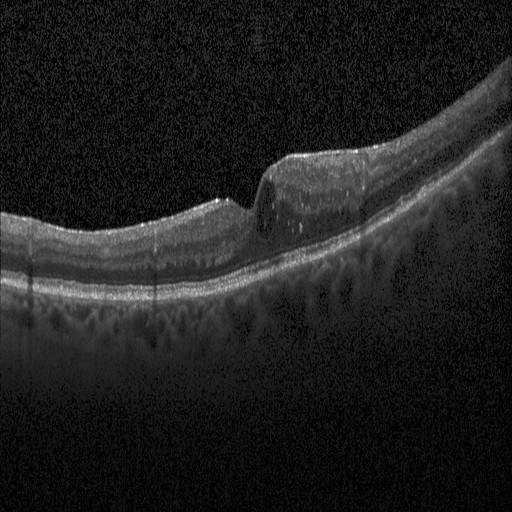
Impression: diabetic macular edema (DME).